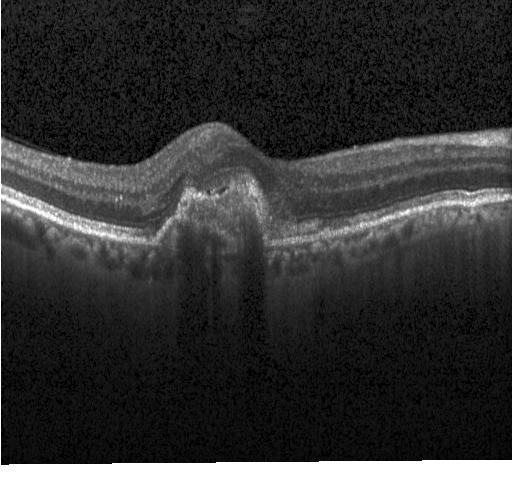

Diagnosis: CNV.